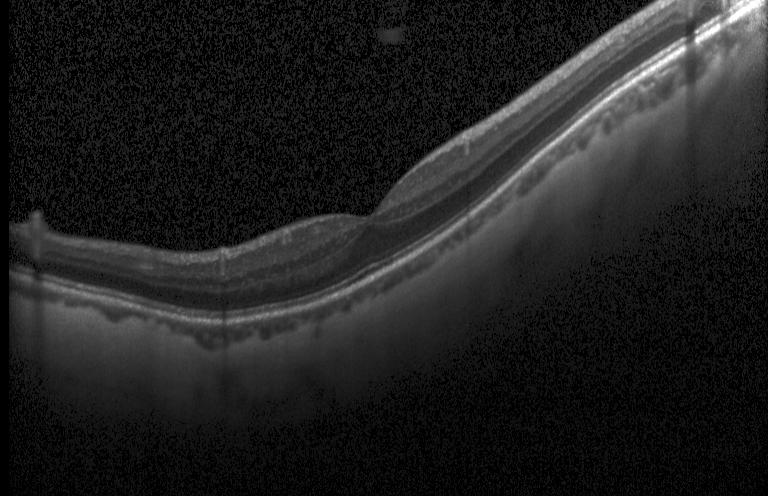 Horizontal scan through the fovea; spectral-domain OCT; OCT B-scan. No choroidal neovascularization, diabetic macular edema, or drusen.